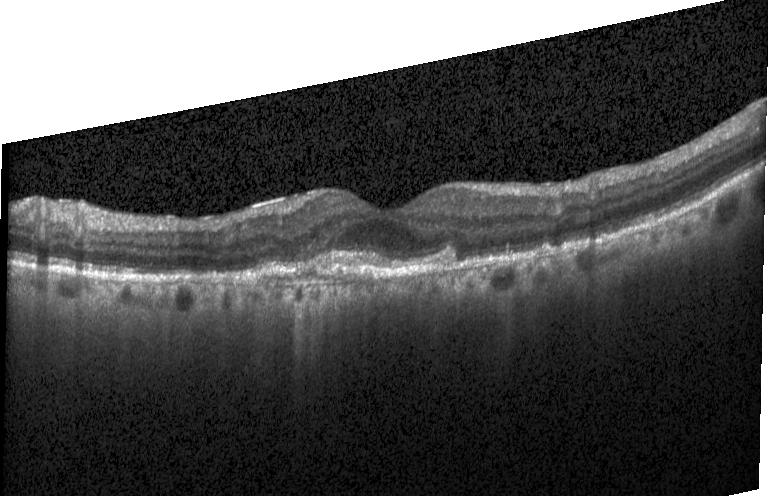 OCT scan showing CNV.